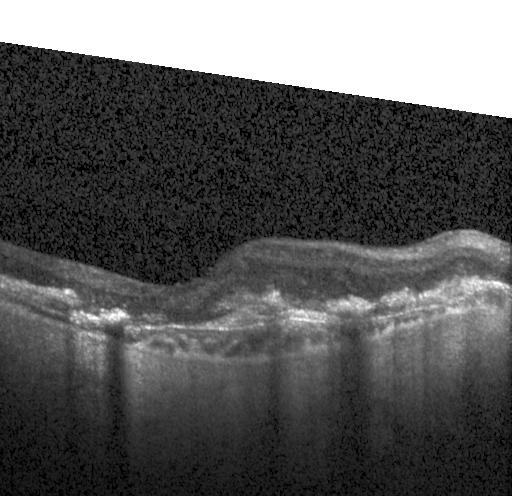

Optical coherence tomography B-scan — CNV.